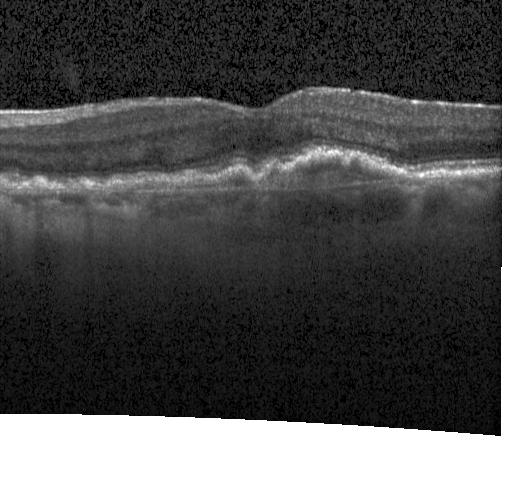
Heidelberg Spectralis · optical coherence tomography B-scan · horizontal scan through the fovea · SD-OCT
The scan shows a choroidal neovascular membrane.